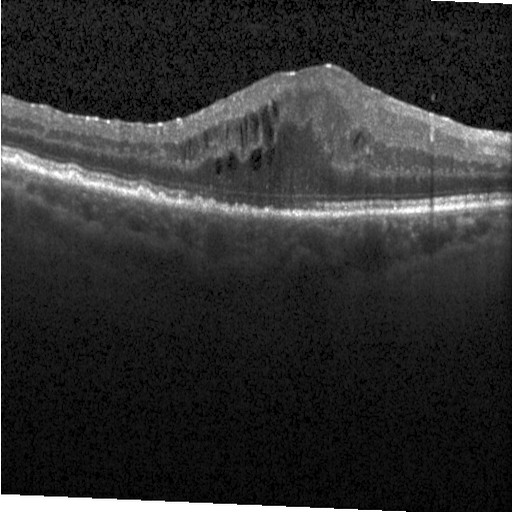 Centered on the fovea. Spectral-domain OCT. Optical coherence tomography B-scan. Heidelberg Spectralis OCT system
Impression: diabetic macular edema.